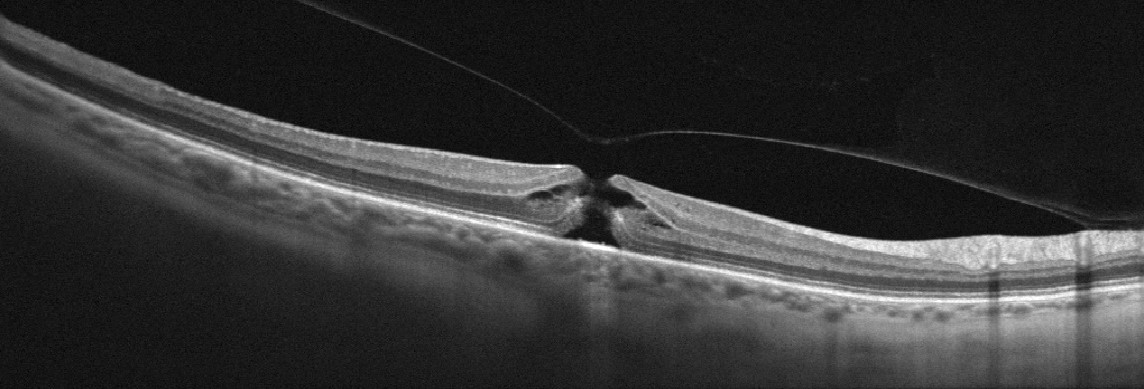

OCT line scan. Fovea-centered
Diagnosis: vitreomacular interface disease (VID).